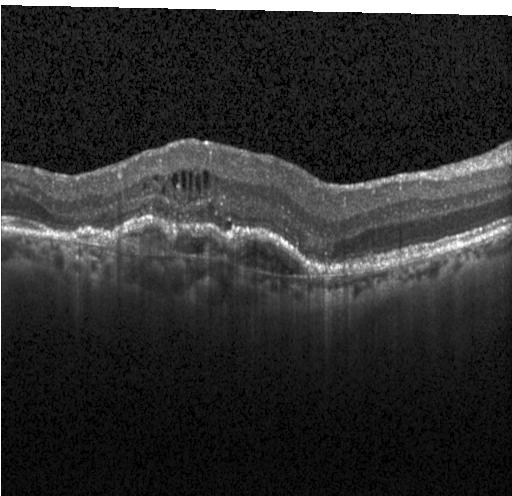

OCT scan showing a choroidal neovascular membrane.